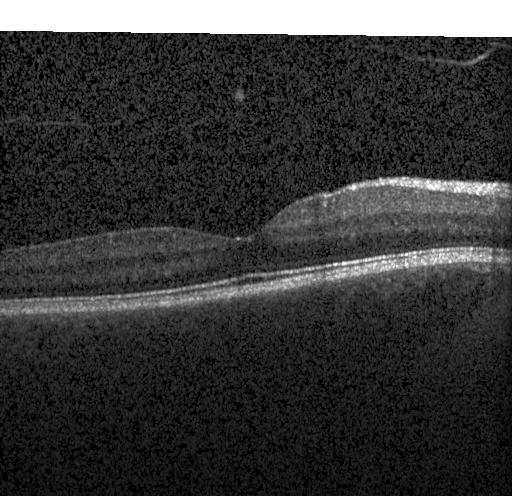

Horizontal scan through the fovea; SD-OCT; optical coherence tomography B-scan
Finding: no evidence of choroidal neovascularization, diabetic macular edema, or drusen.